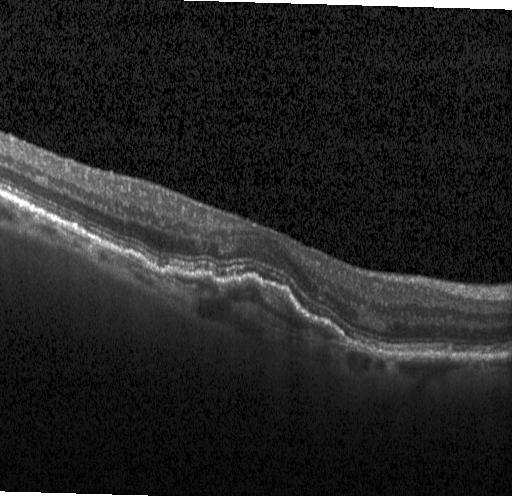

Macular OCT: a choroidal neovascular membrane.